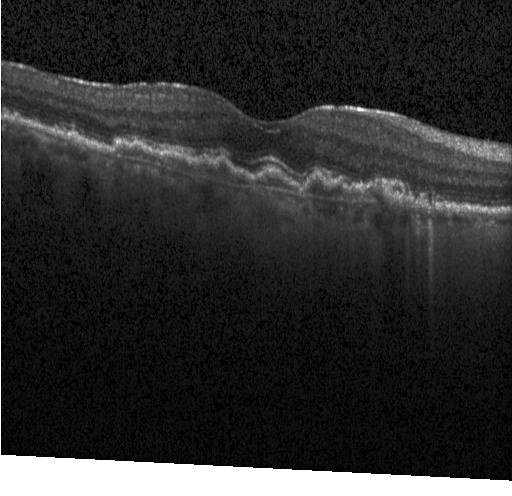 Macular OCT demonstrating CNV.